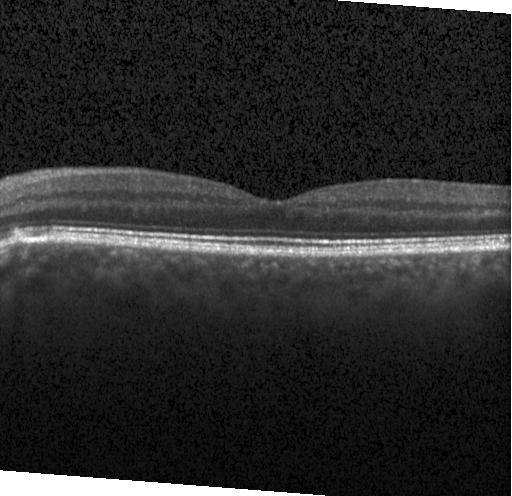 Spectral-domain OCT B-scan: neither choroidal neovascularization, diabetic macular edema, nor drusen.